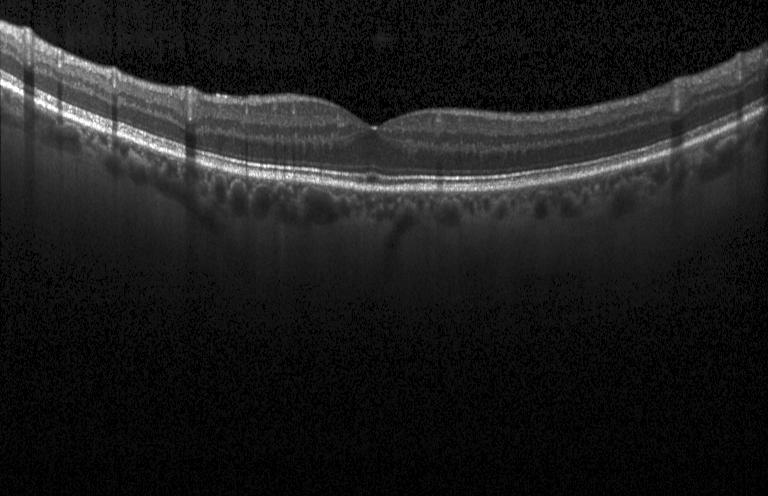
Macular OCT demonstrating no evidence of choroidal neovascularization, diabetic macular edema, or drusen.